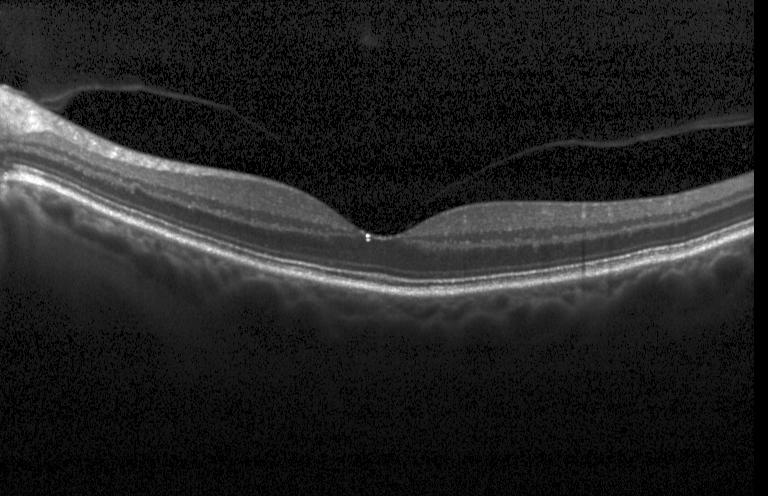

Optical coherence tomography B-scan.
Diagnosis: no choroidal neovascularization, no diabetic macular edema, and no drusen.